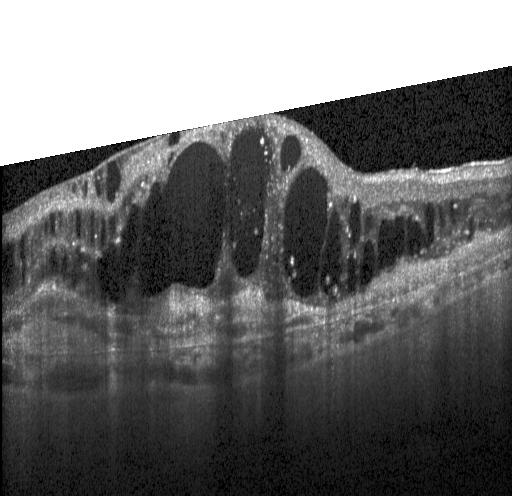 Spectral-domain OCT, macular scan, Heidelberg Spectralis, retinal OCT B-scan — Impression: a choroidal neovascular membrane.